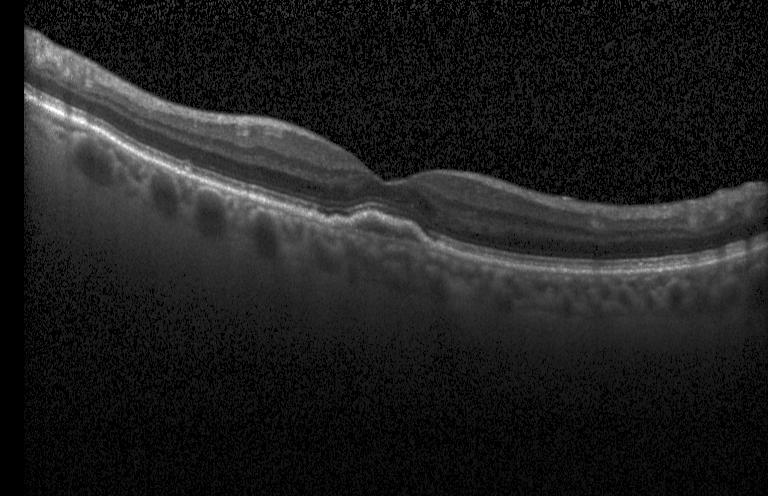

Dx: a choroidal neovascular membrane.